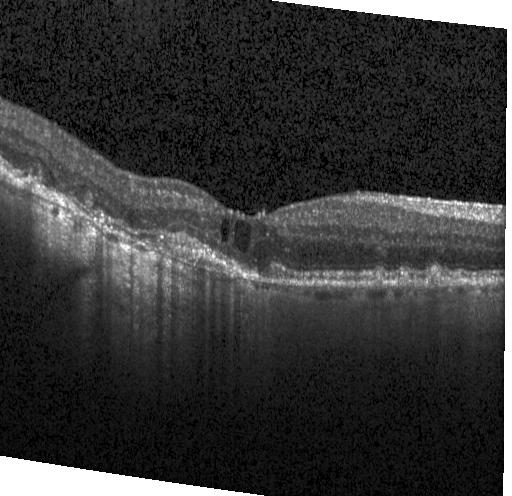
The scan shows CNV.